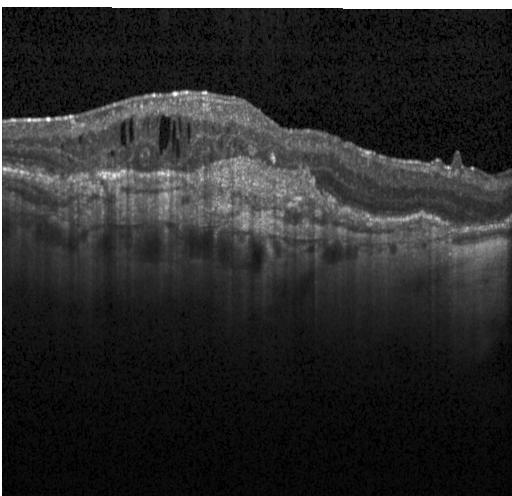 Spectral-domain OCT B-scan: a choroidal neovascular membrane.